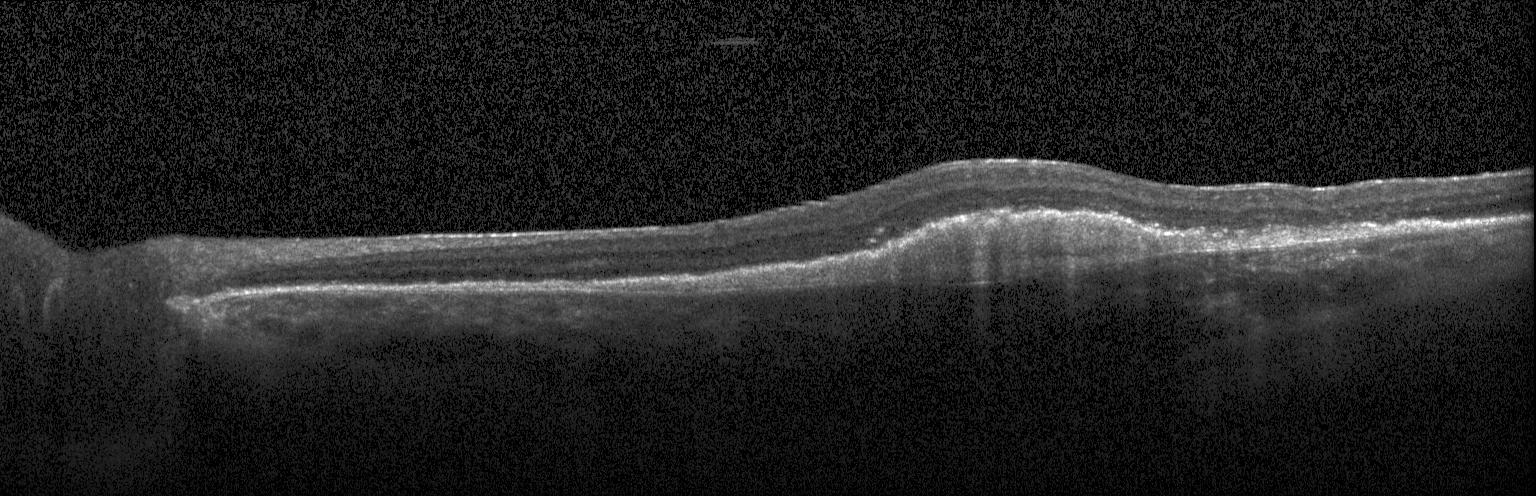
Macular OCT demonstrating CNV.